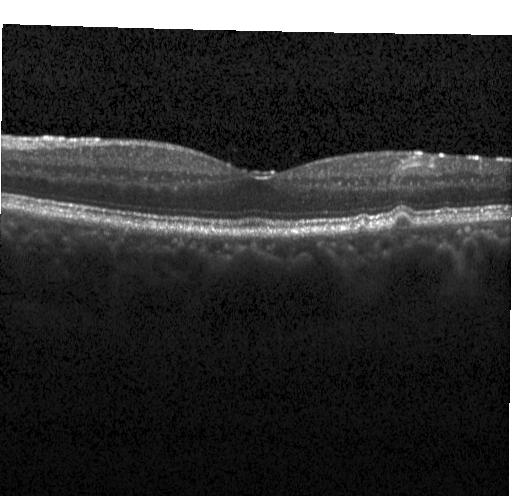

OCT scan showing multiple drusen.